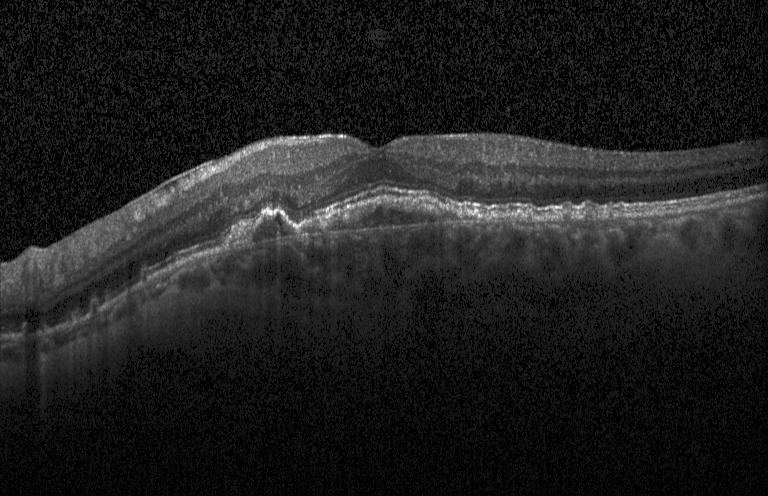
Spectral-domain optical coherence tomography, retinal OCT B-scan, macular scan. Diagnosis: CNV.